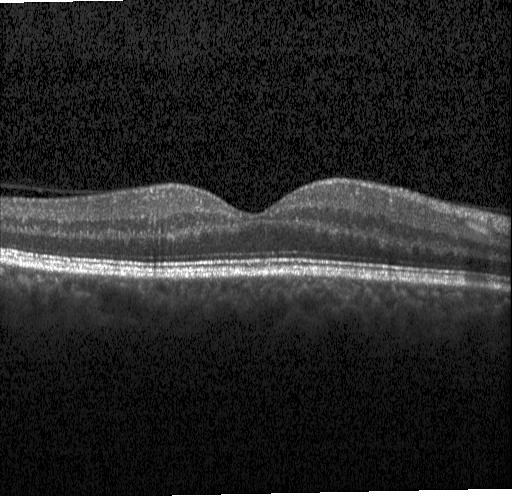 Spectral-domain optical coherence tomography · fovea-centered · Heidelberg Spectralis OCT system · OCT line scan
Dx: neither choroidal neovascularization, diabetic macular edema, nor drusen.